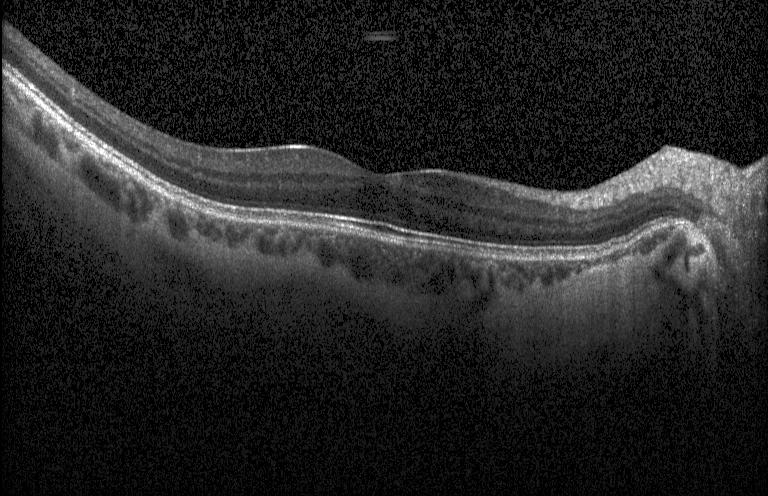
Optical coherence tomography B-scan. Horizontal scan through the fovea.
Diagnosis: neither choroidal neovascularization, diabetic macular edema, nor drusen.